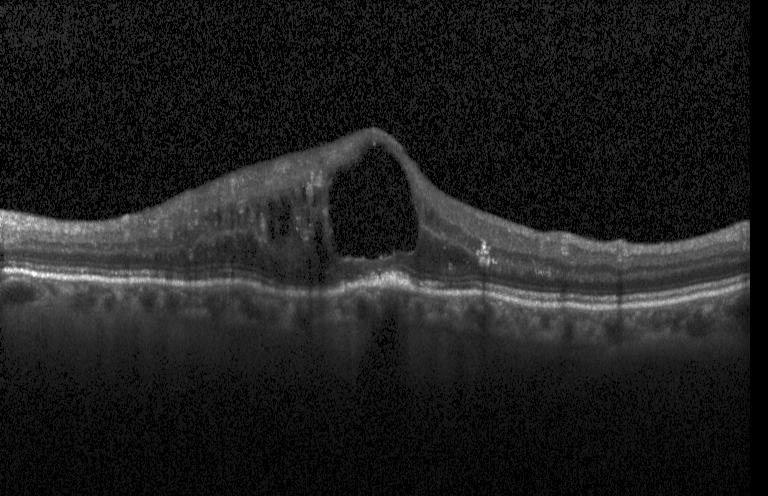
Horizontal scan through the fovea. OCT B-scan. Acquired on a Heidelberg Spectralis. Spectral-domain OCT.
Impression: diabetic macular edema (DME).